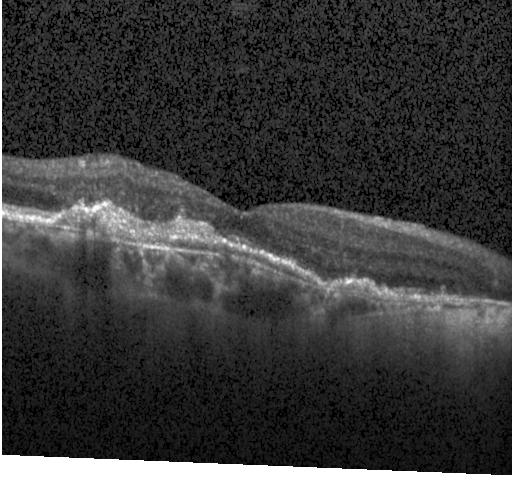

Macular OCT demonstrating a choroidal neovascular membrane.